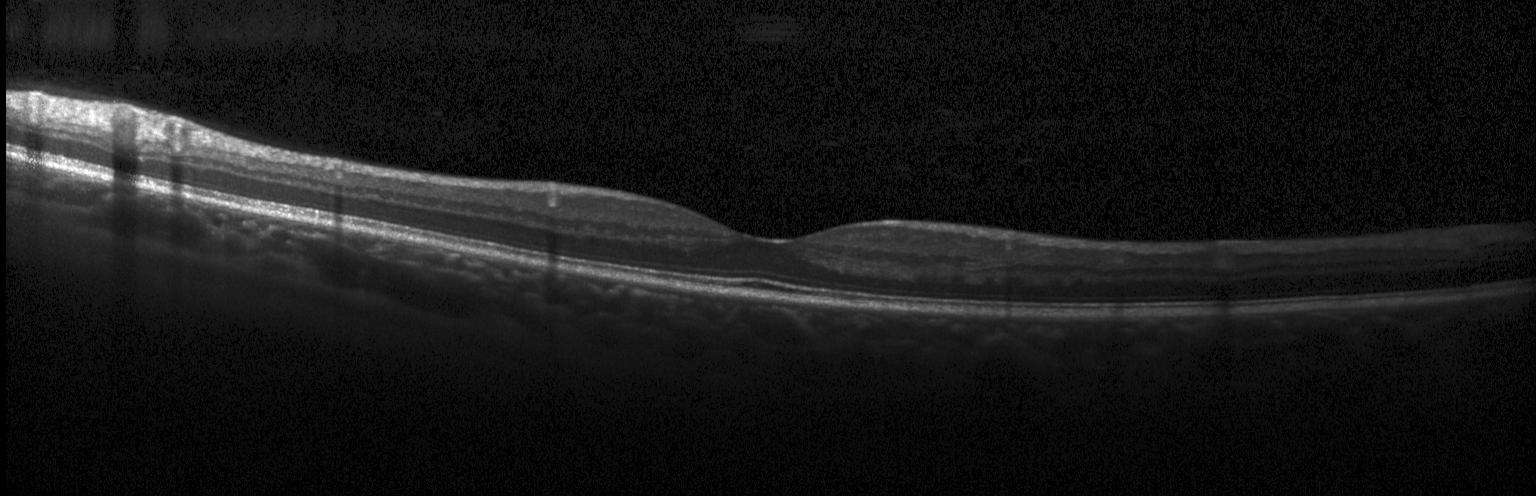
Acquired on a Heidelberg Spectralis, SD-OCT, centered on the fovea, optical coherence tomography scan. Impression: no evidence of CNV, DME, or drusen.